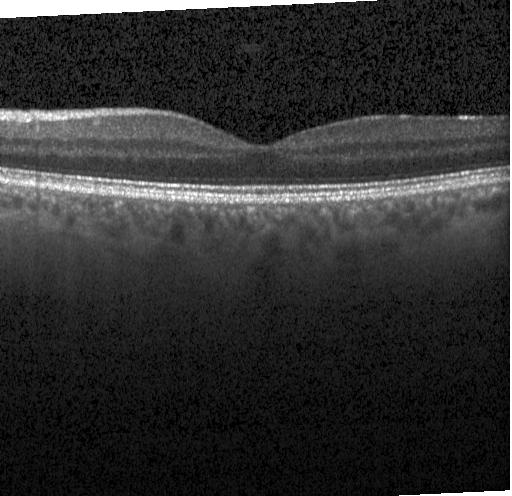
Fovea-centered. Heidelberg Spectralis. Spectral-domain optical coherence tomography. Retinal OCT cross-section — Finding: no CNV, no DME, and no drusen.